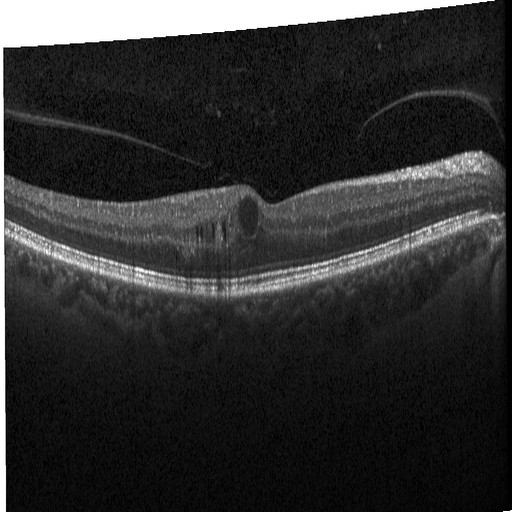 Diagnosis: diabetic macular edema.